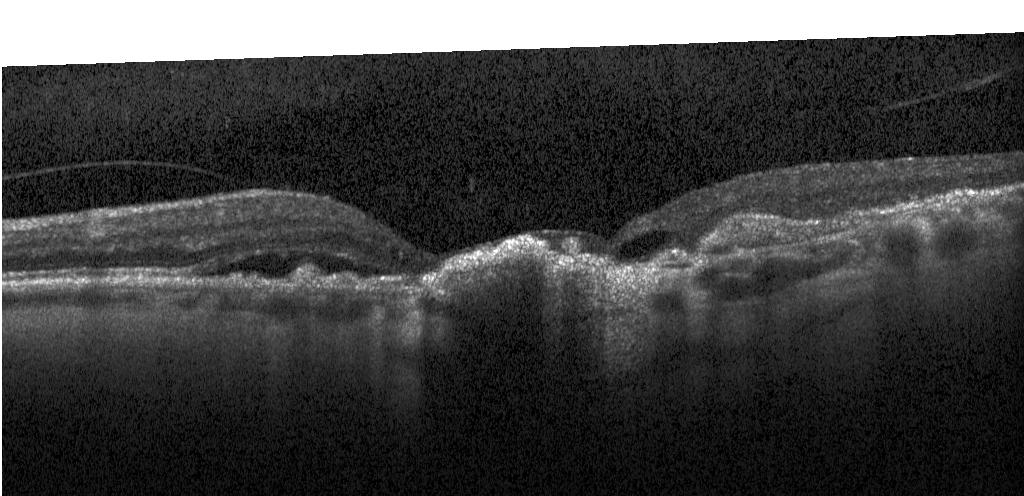
OCT B-scan.
Assessment: a choroidal neovascular membrane.